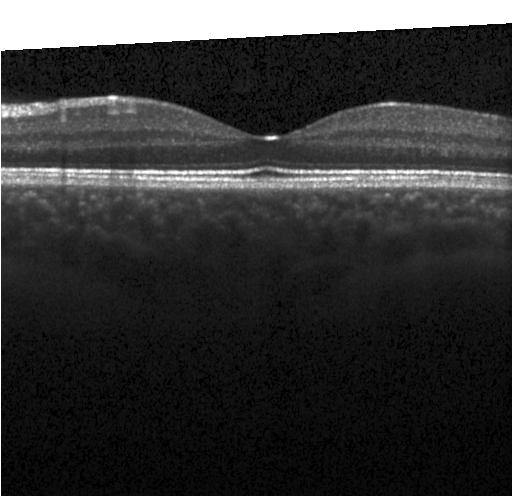 Acquired on a Heidelberg Spectralis. Optical coherence tomography B-scan.
The scan shows neither CNV, DME, nor drusen.